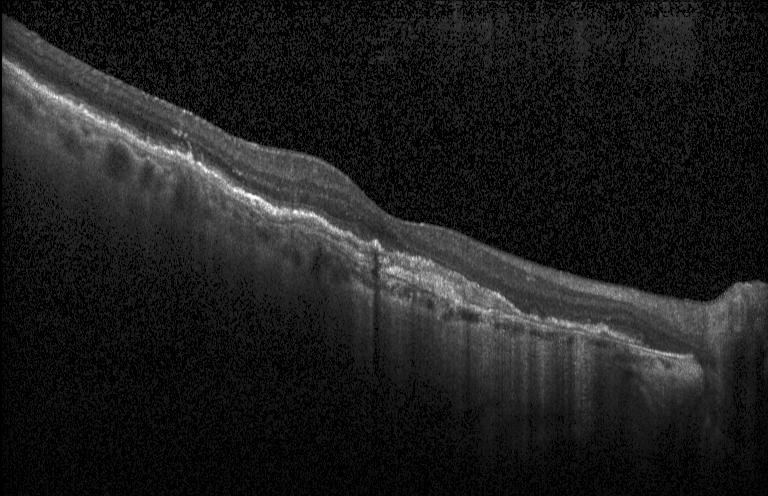
Retinal OCT cross-section; spectral-domain optical coherence tomography; centered on the fovea.
The scan shows choroidal neovascularization.